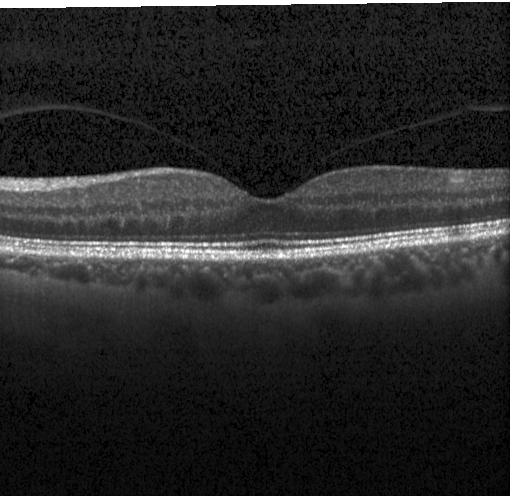
OCT B-scan. This B-scan demonstrates no choroidal neovascularization, diabetic macular edema, or drusen.